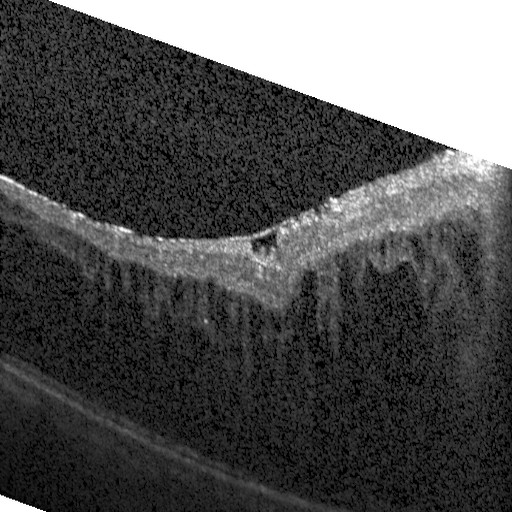

Macular OCT: DME.